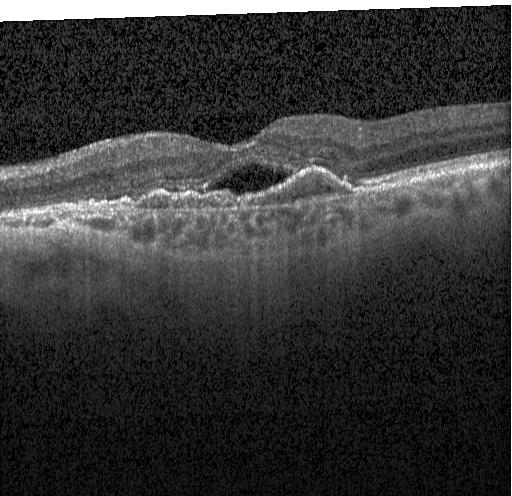 OCT B-scan
The scan shows choroidal neovascularization (CNV).